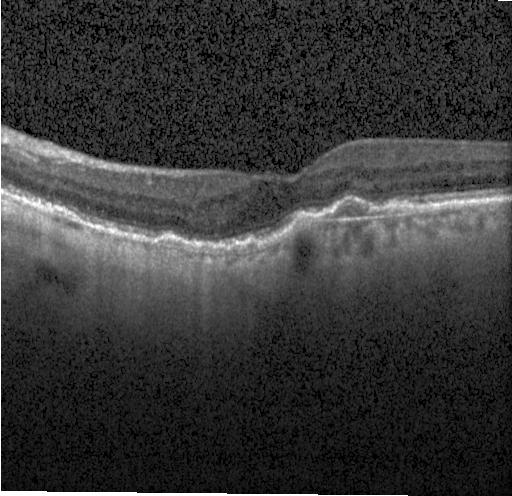

Retinal OCT B-scan. SD-OCT — The scan shows choroidal neovascularization (CNV).